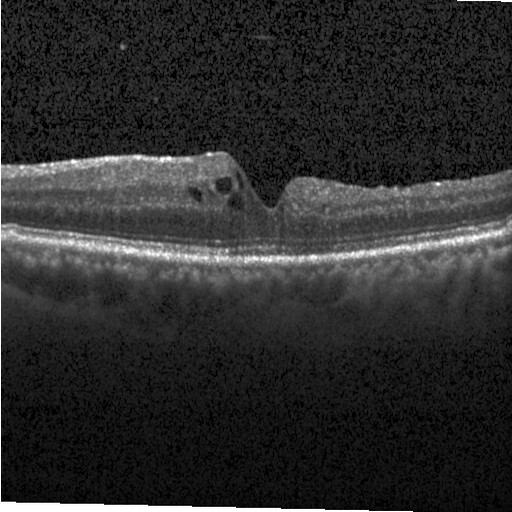

Retinal OCT cross-section — Diagnosis: DME.